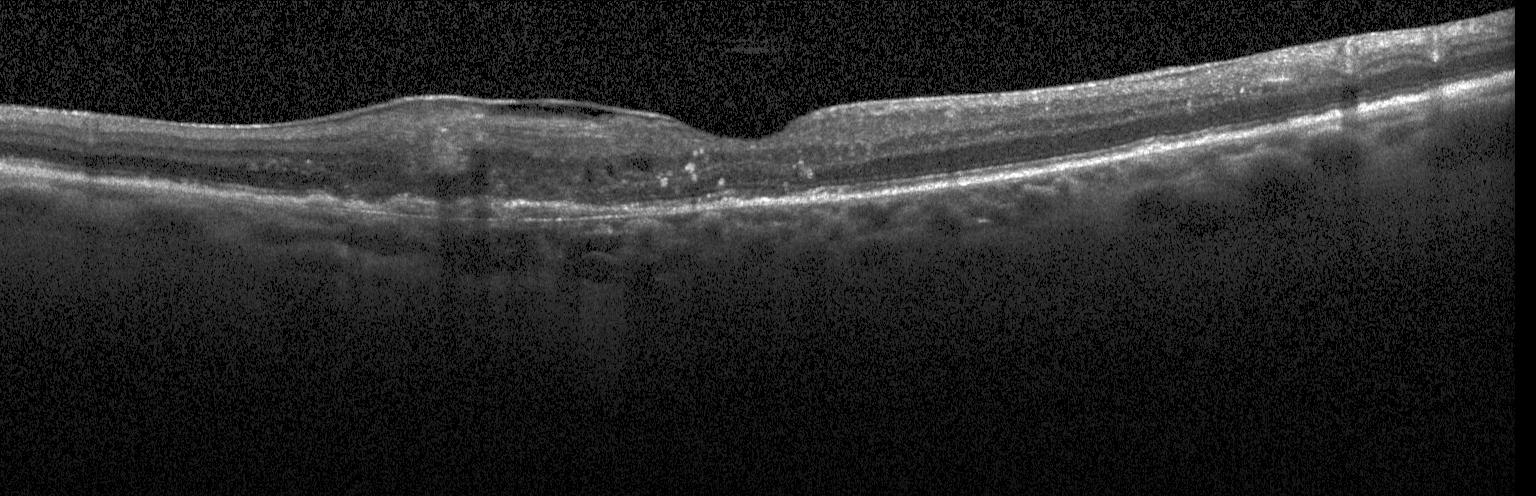 Optical coherence tomography scan — Impression: choroidal neovascularization (CNV).